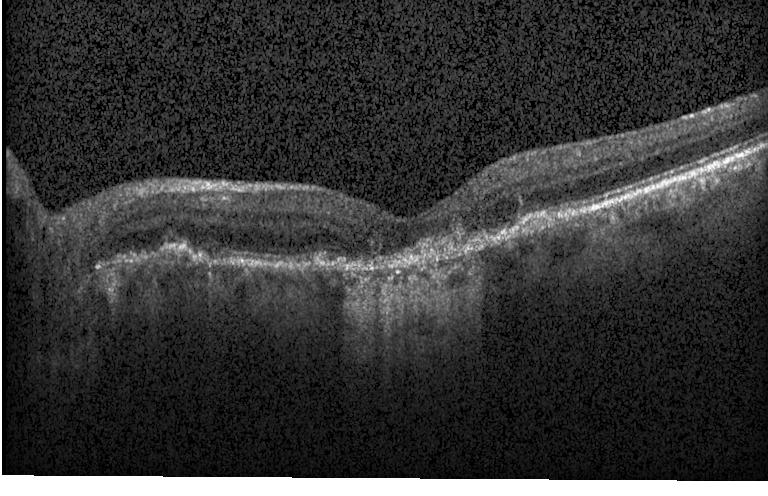 OCT finding: a choroidal neovascular membrane.